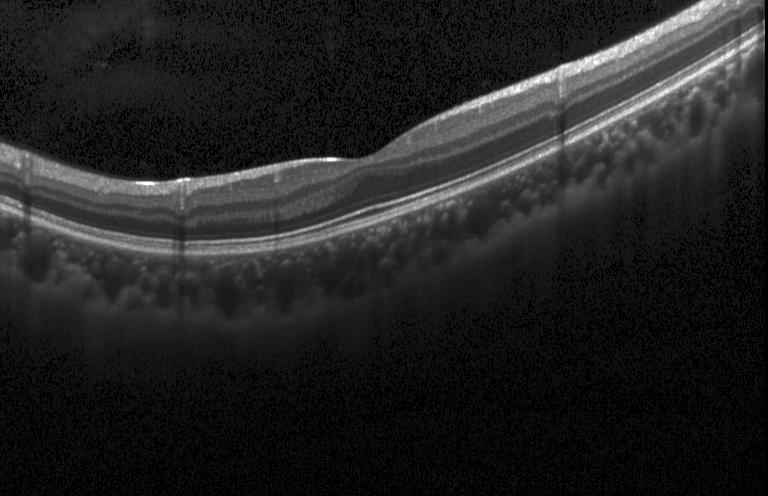 No choroidal neovascularization, no diabetic macular edema, and no drusen.